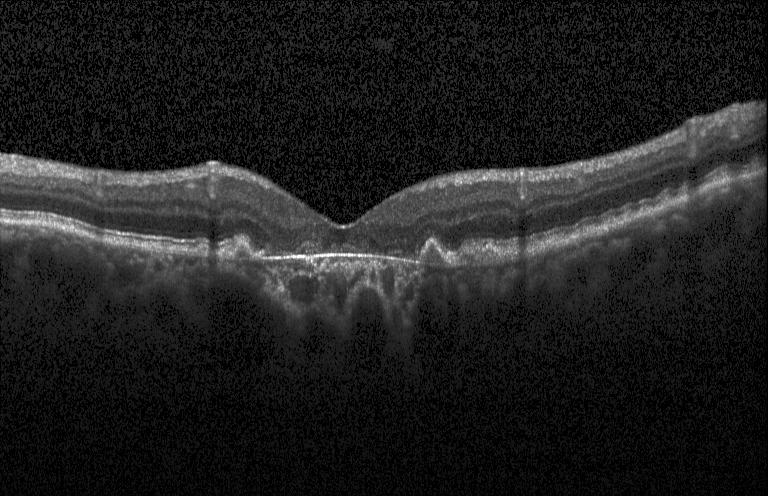
SD-OCT. OCT line scan. Macular OCT: choroidal neovascularization.